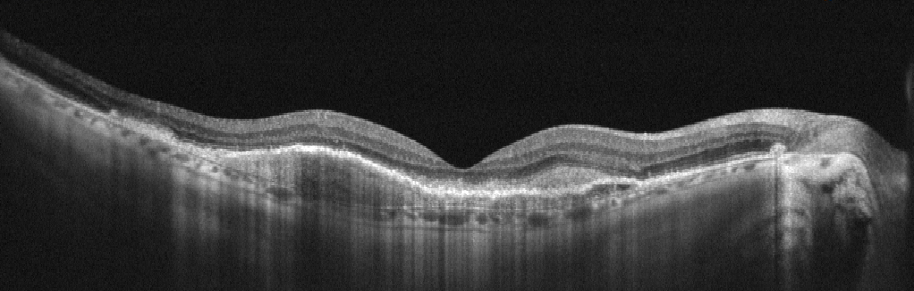 Retinal OCT cross-section. Right eye.
Diagnosis: age-related macular degeneration.